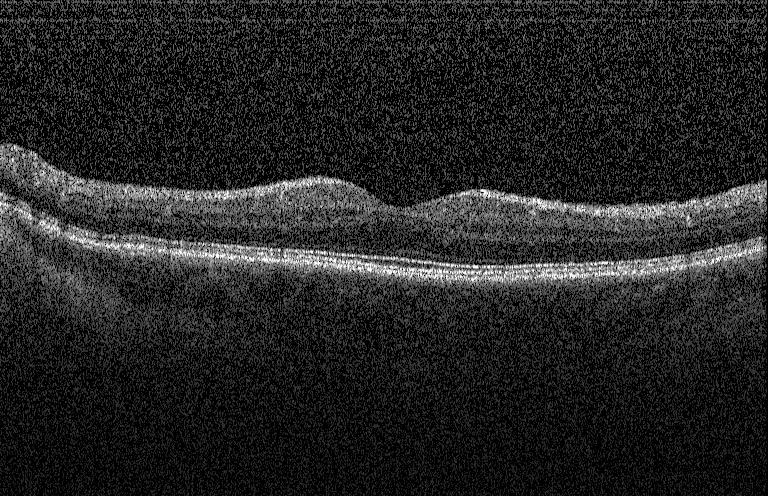 Dx: no CNV, DME, or drusen.